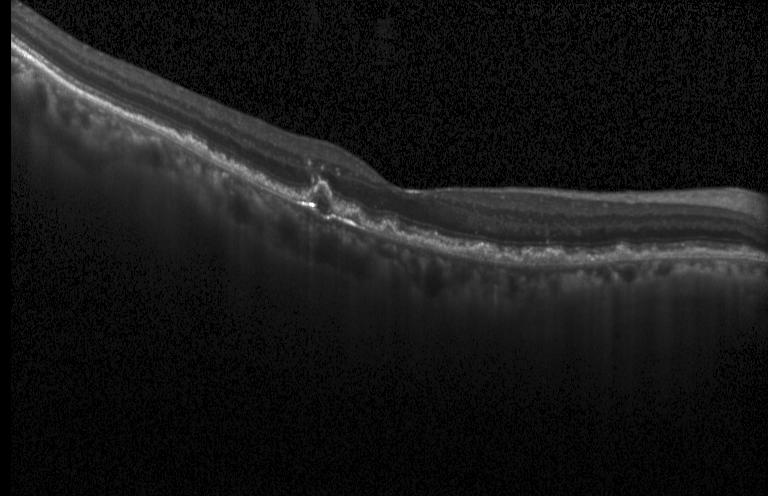 Heidelberg Spectralis, optical coherence tomography B-scan.
Impression: a choroidal neovascular membrane.